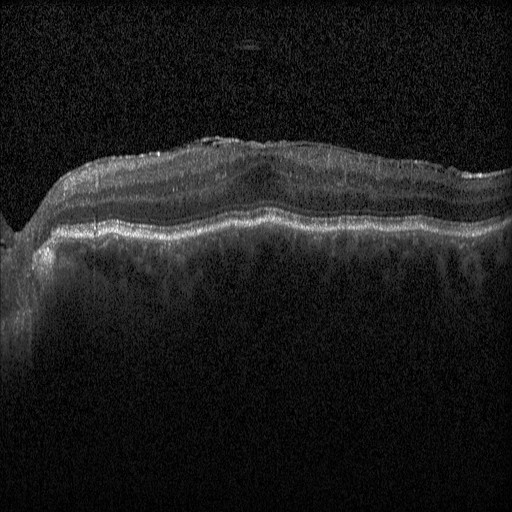 OCT B-scan showing DME.